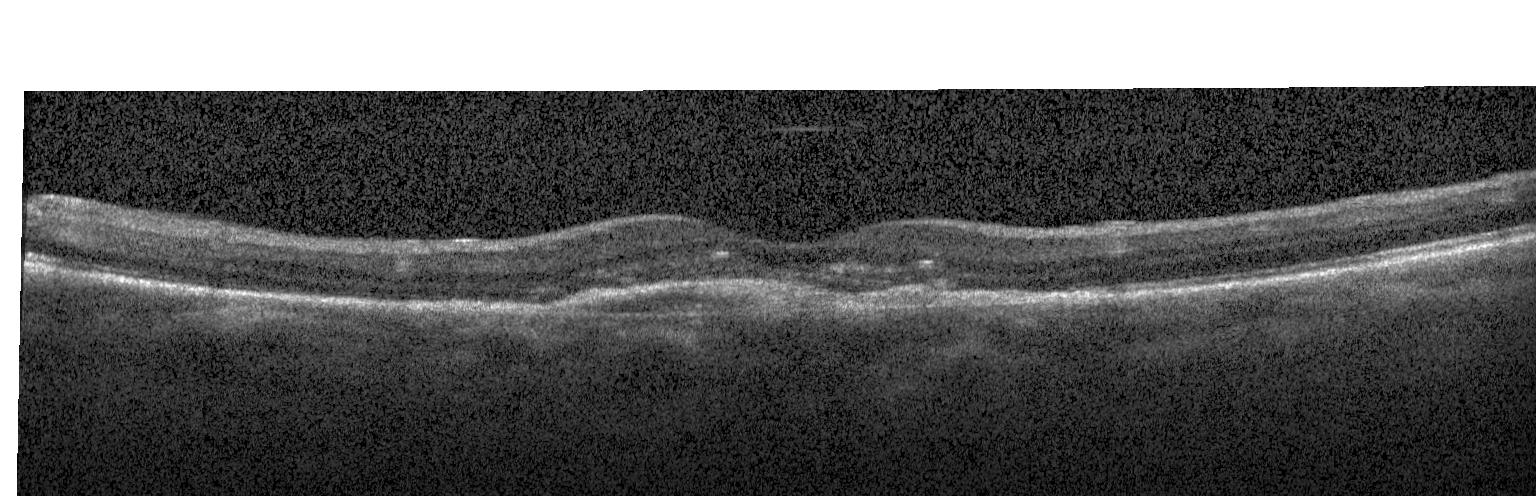
Impression: CNV.